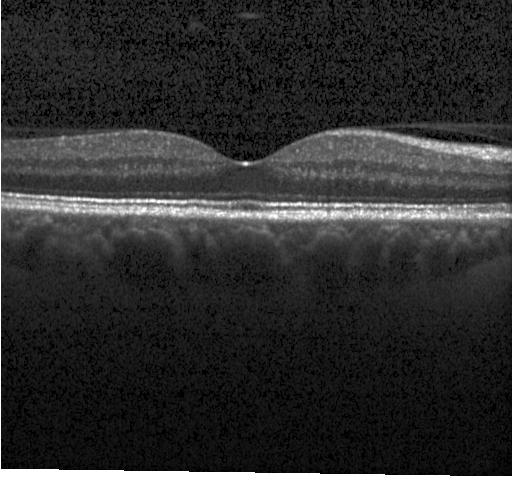

OCT scan showing no choroidal neovascularization, diabetic macular edema, or drusen.